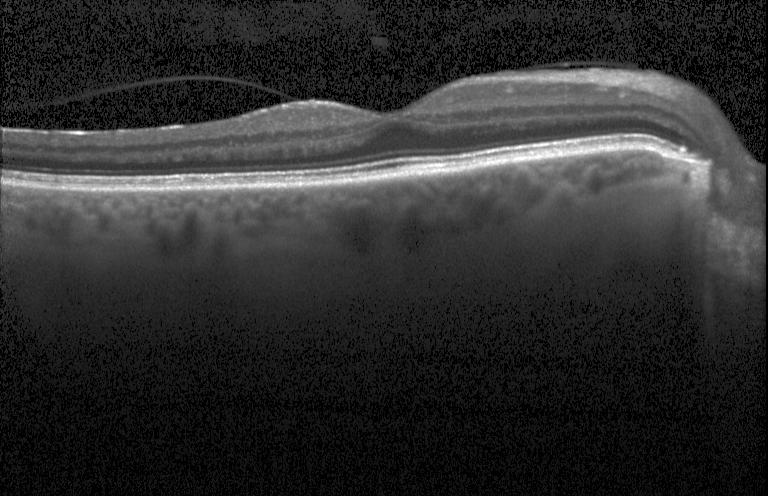 Fovea-centered, retinal OCT B-scan, Heidelberg Spectralis OCT system — Finding: no choroidal neovascularization, diabetic macular edema, or drusen.